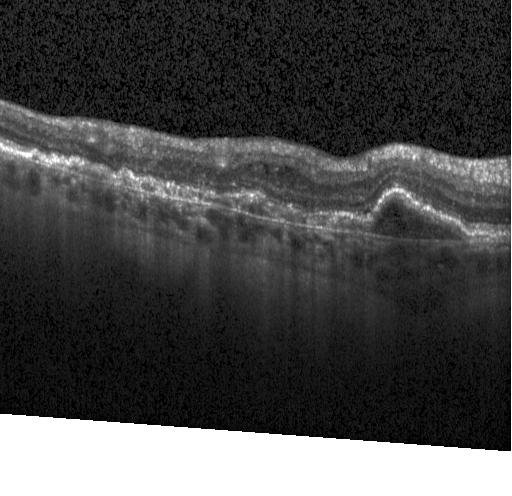 OCT scan showing choroidal neovascularization.